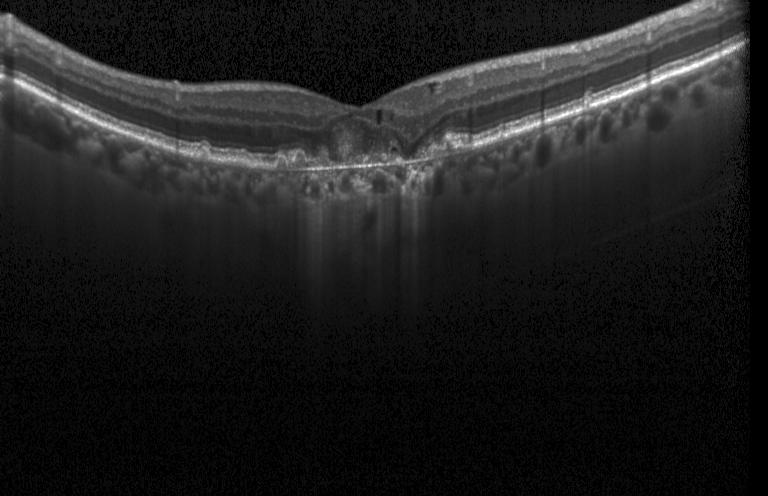 OCT B-scan. Diagnosis: choroidal neovascularization.